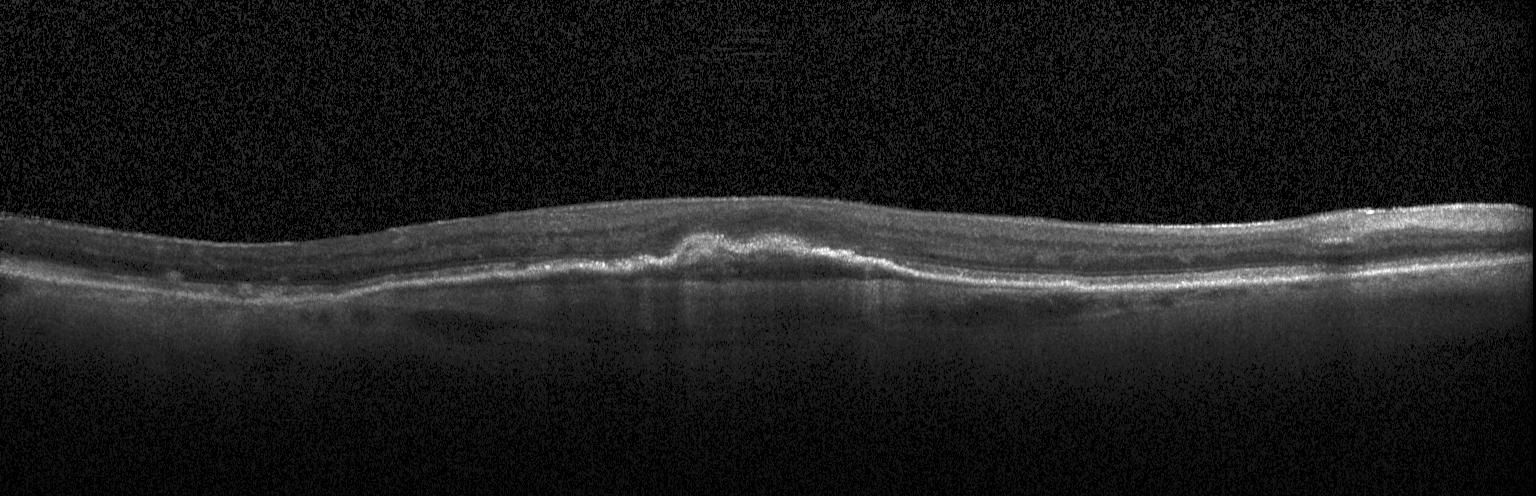 Macular OCT demonstrating a choroidal neovascular membrane.